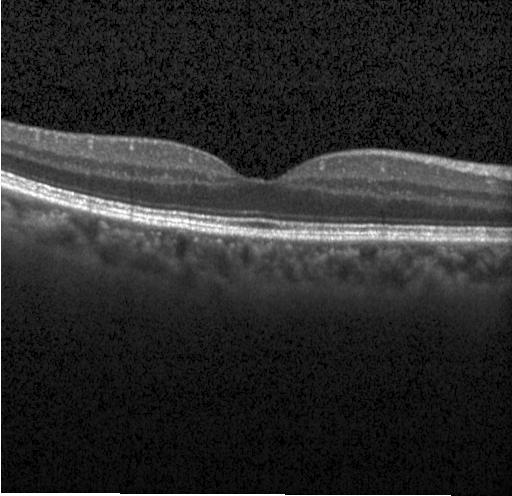
Dx: neither CNV, DME, nor drusen.